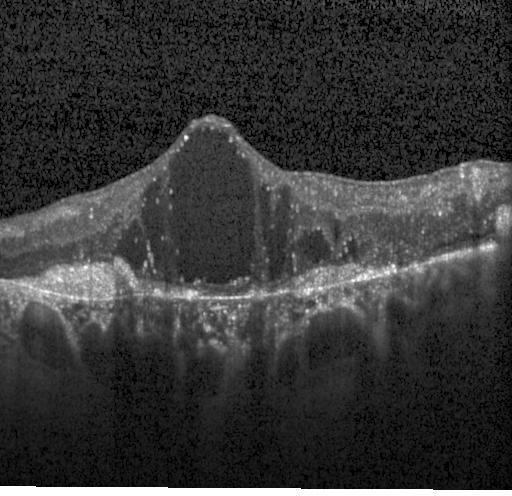

OCT B-scan, macular scan, SD-OCT — Diagnosis: a choroidal neovascular membrane.